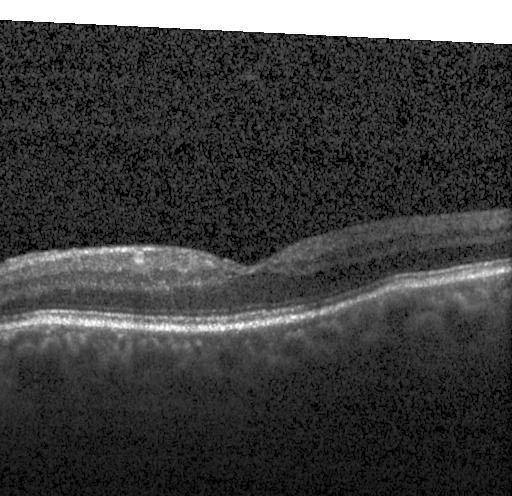 Diagnosis: no evidence of choroidal neovascularization, diabetic macular edema, or drusen.